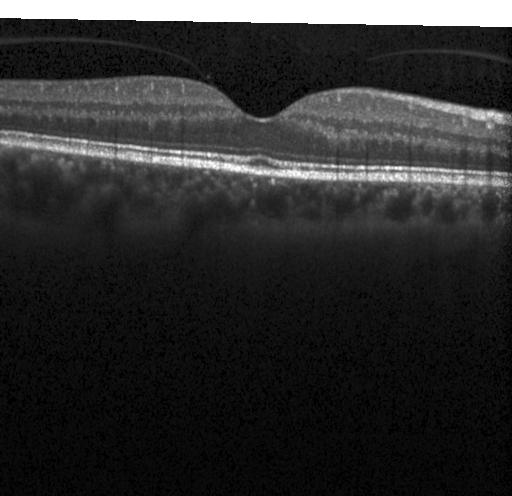

Retinal OCT cross-section.
No choroidal neovascularization, no diabetic macular edema, and no drusen.